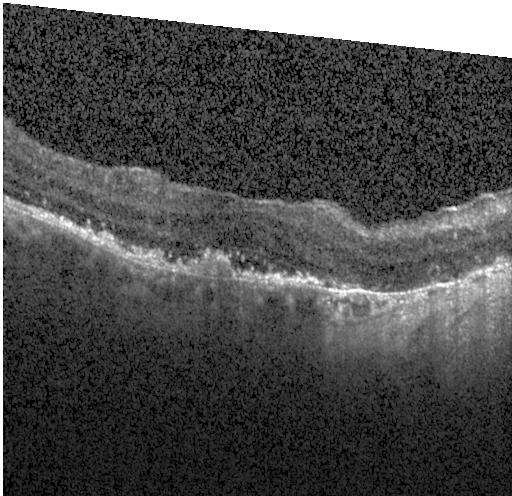
Fovea-centered; SD-OCT; retinal OCT cross-section; instrument: Heidelberg Spectralis
The scan shows choroidal neovascularization.